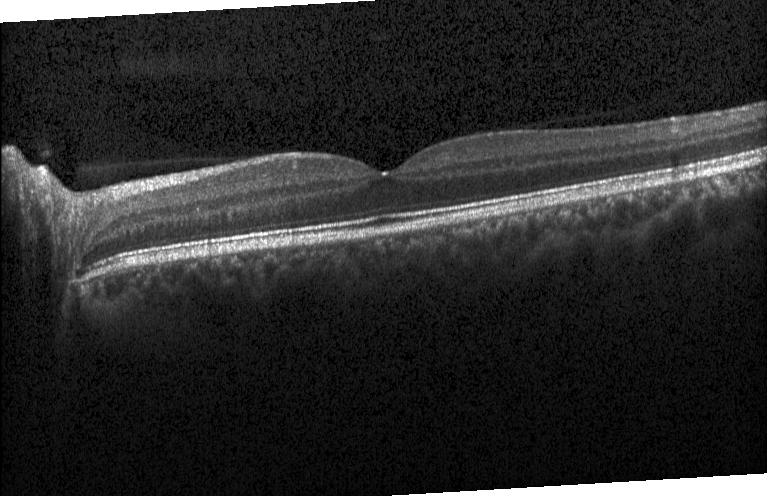 Optical coherence tomography B-scan, fovea-centered, Heidelberg Spectralis.
Macular OCT: neither choroidal neovascularization, diabetic macular edema, nor drusen.